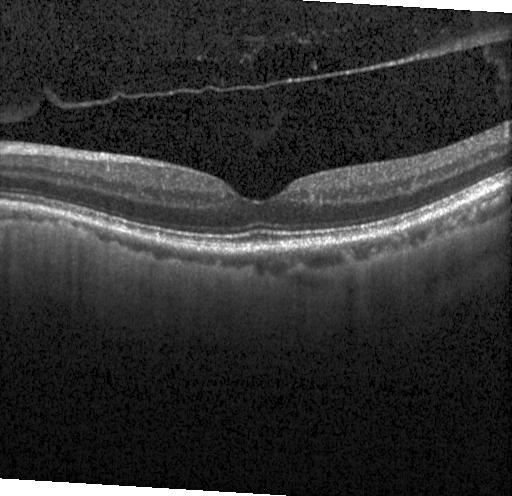

Dx: no choroidal neovascularization, no diabetic macular edema, and no drusen.